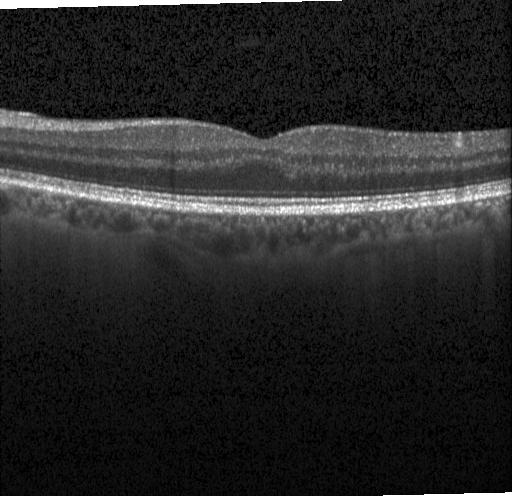
Diagnosis: no choroidal neovascularization, diabetic macular edema, or drusen.